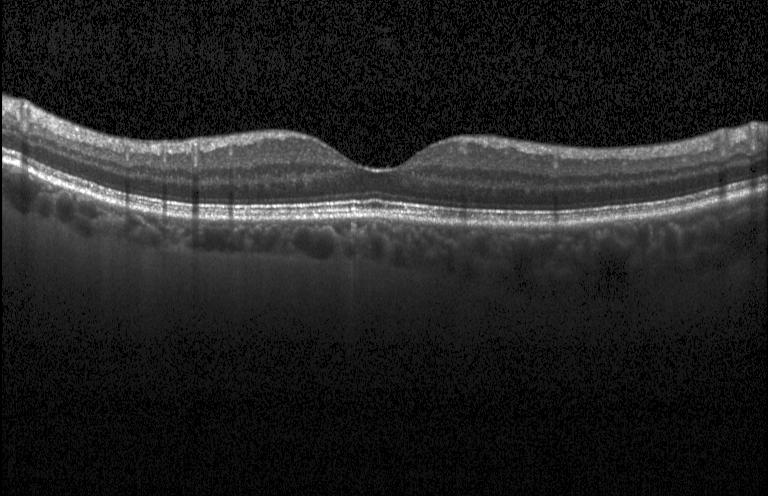
Horizontal scan through the fovea. Spectral-domain optical coherence tomography. Heidelberg Spectralis OCT system. OCT B-scan
OCT finding: no CNV, no DME, and no drusen.